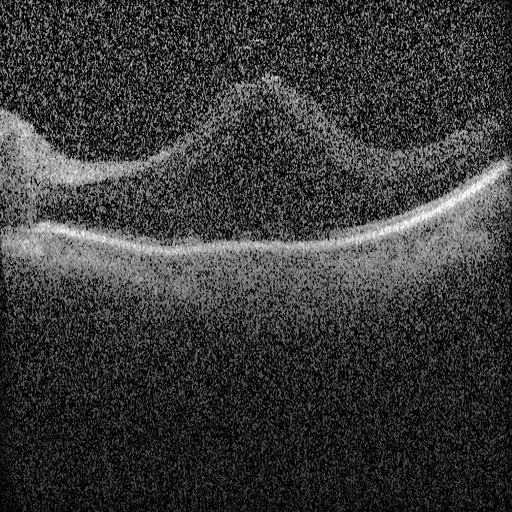
Optical coherence tomography B-scan; through the macula. Diagnosis: DME.